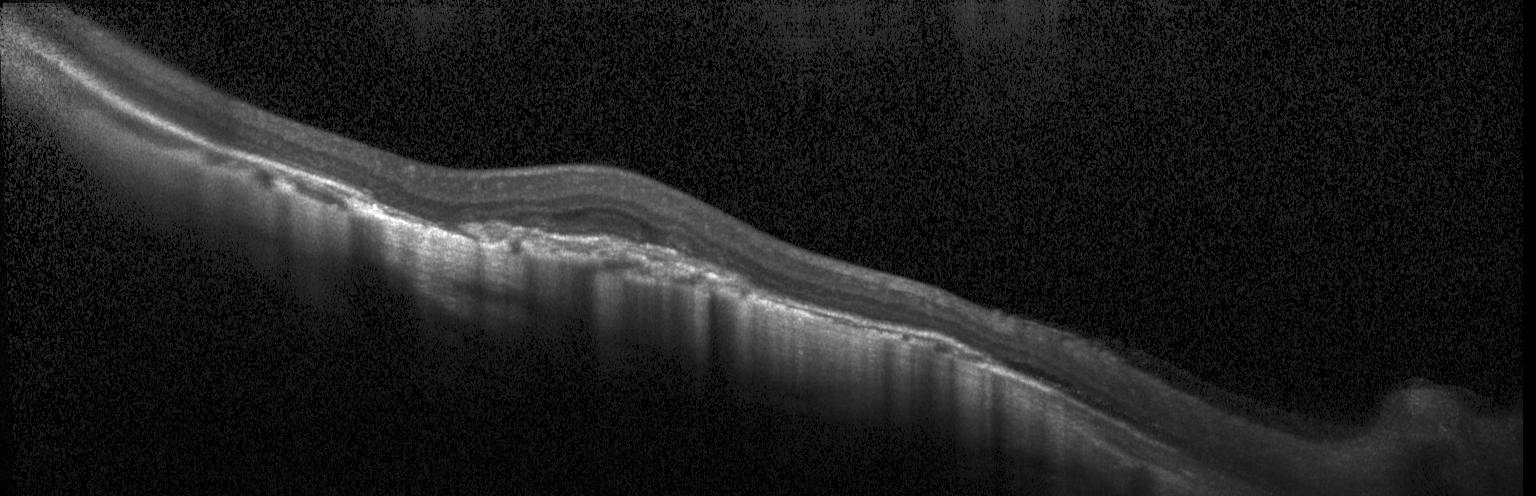
OCT B-scan showing choroidal neovascularization (CNV).